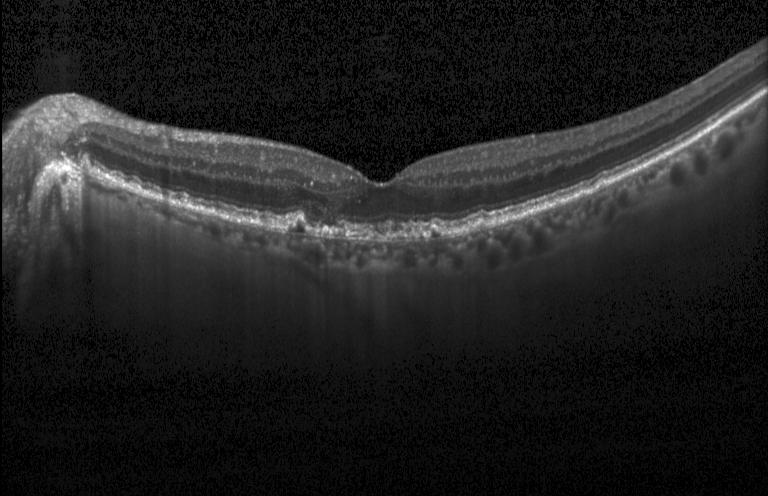 Dx: drusen.